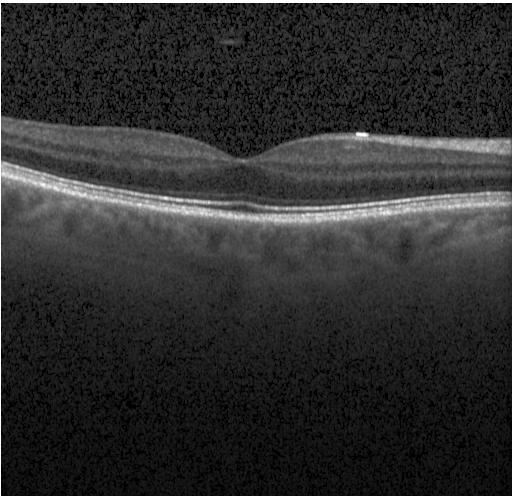

OCT scan showing no choroidal neovascularization, diabetic macular edema, or drusen.